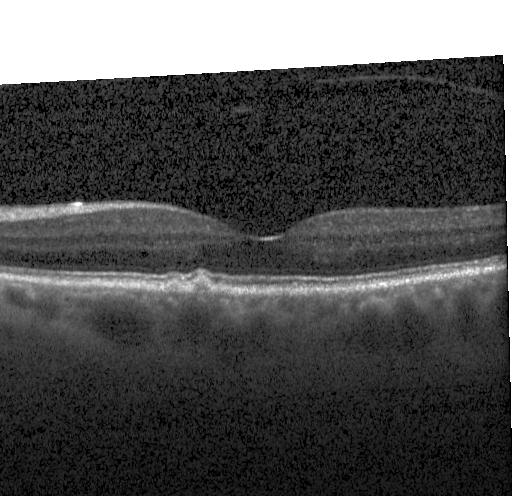
Diagnosis: sub-RPE drusenoid deposits.